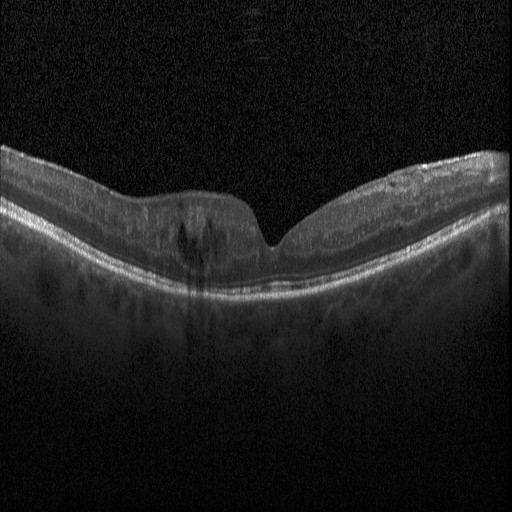

Retinal OCT cross-section showing DME.